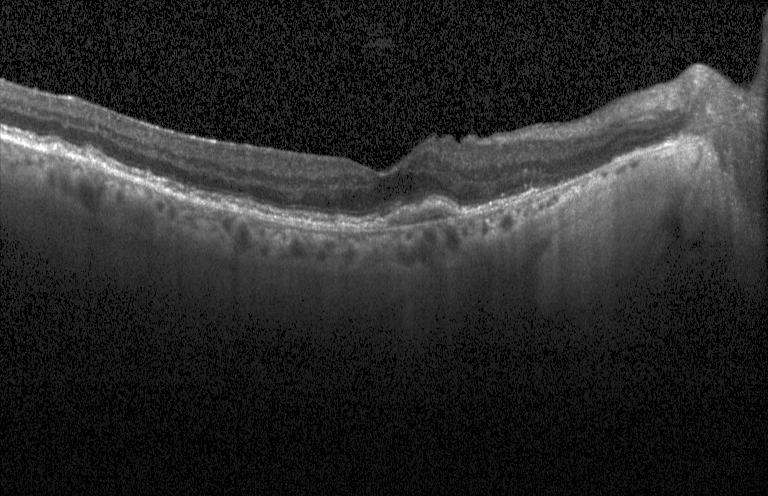
Centered on the fovea. Optical coherence tomography scan. Heidelberg Spectralis OCT system. SD-OCT — This B-scan demonstrates a choroidal neovascular membrane.